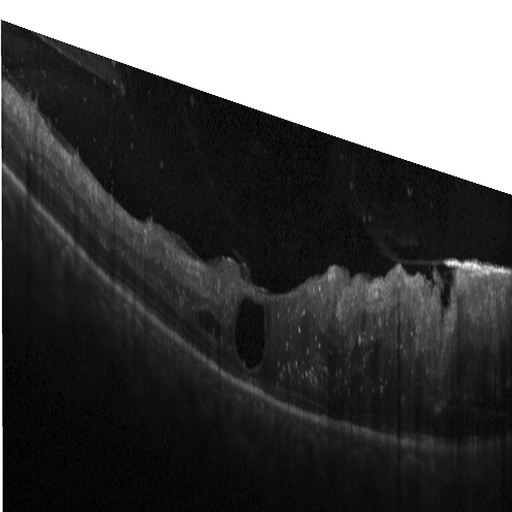 Retinal OCT B-scan.
Impression: diabetic macular edema.